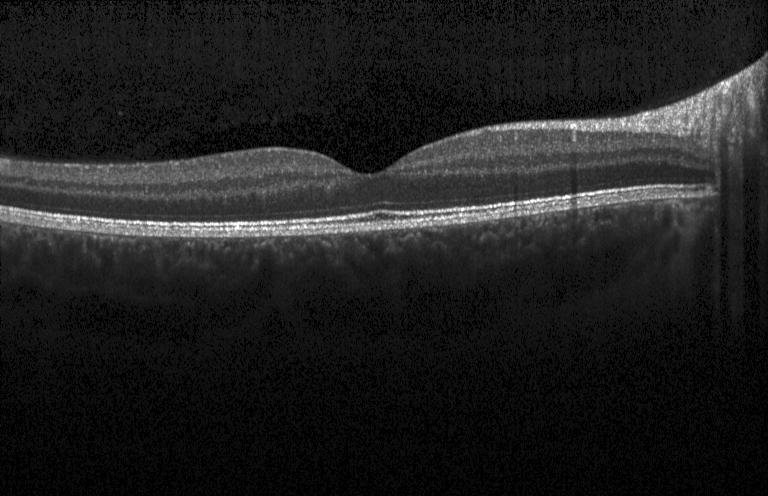
Optical coherence tomography scan — Impression: no evidence of choroidal neovascularization, diabetic macular edema, or drusen.